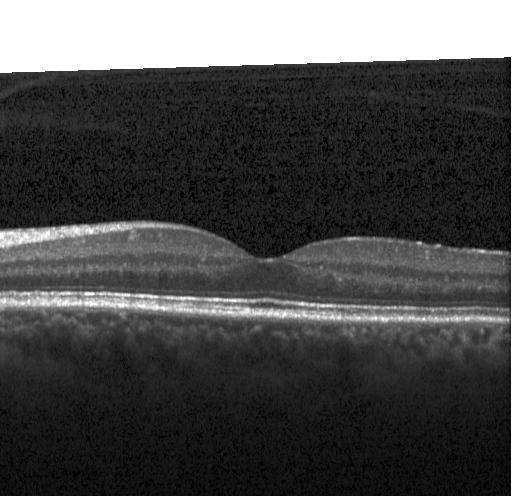 Retinal OCT B-scan; macular scan; spectral-domain OCT; instrument: Heidelberg Spectralis.
Impression: no choroidal neovascularization, diabetic macular edema, or drusen.